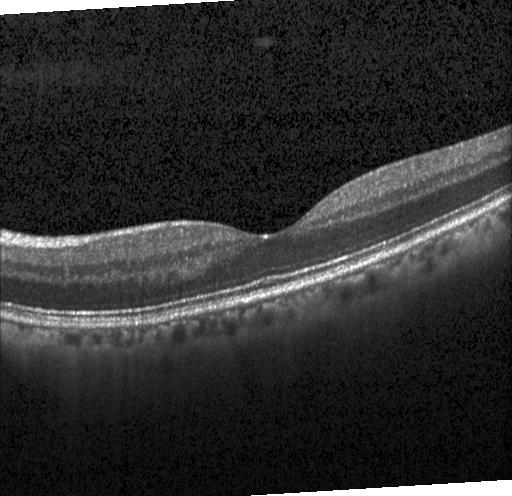 Retinal OCT B-scan · spectral-domain optical coherence tomography · Heidelberg Spectralis OCT system. Diagnosis: no evidence of choroidal neovascularization, diabetic macular edema, or drusen.